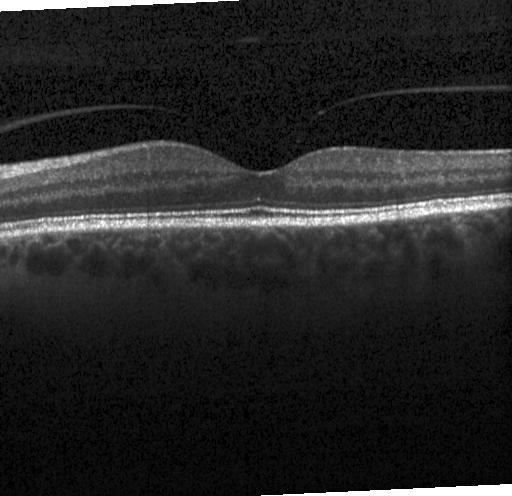 Diagnosis: no CNV, DME, or drusen.